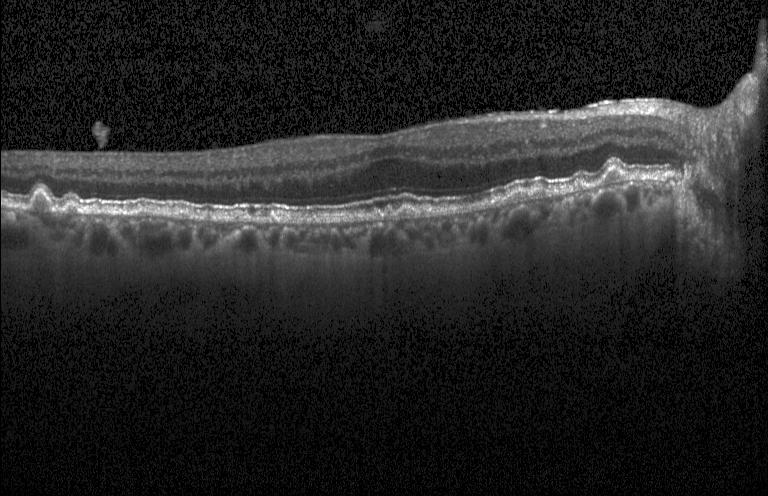

SD-OCT; horizontal scan through the fovea; optical coherence tomography B-scan. Assessment: multiple drusen.